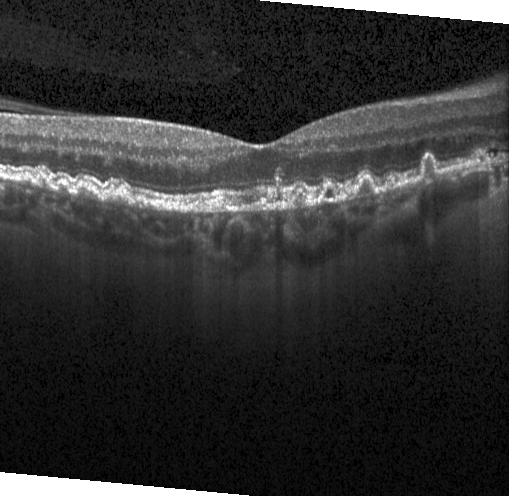 Centered on the fovea. SD-OCT. Optical coherence tomography scan.
Finding: a choroidal neovascular membrane.